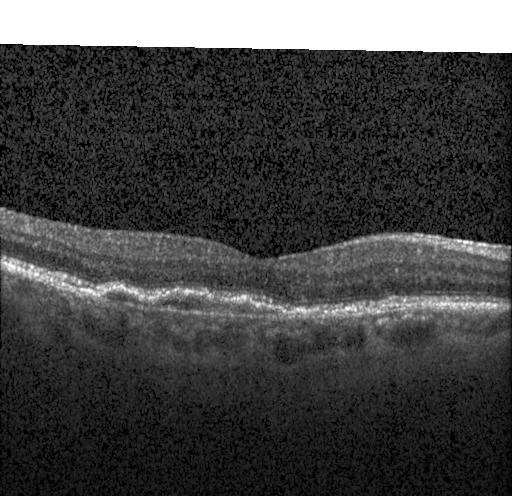

Retinal OCT B-scan. Impression: a choroidal neovascular membrane.